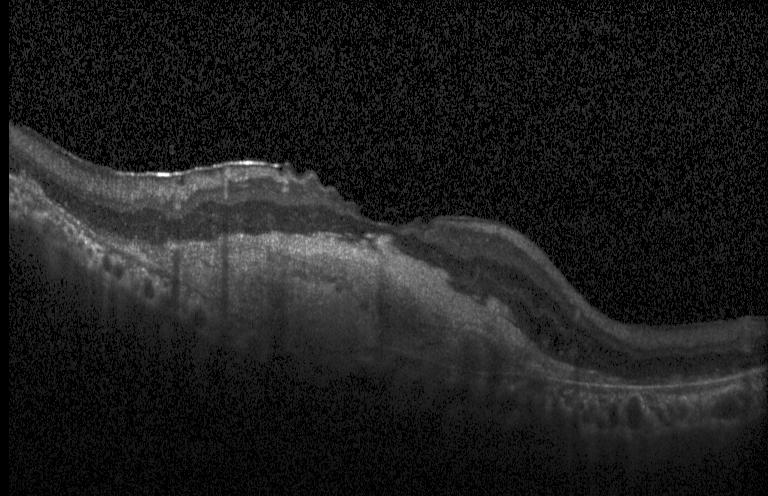
Optical coherence tomography scan. Acquired on a Heidelberg Spectralis. Fovea-centered.
The scan shows a choroidal neovascular membrane.